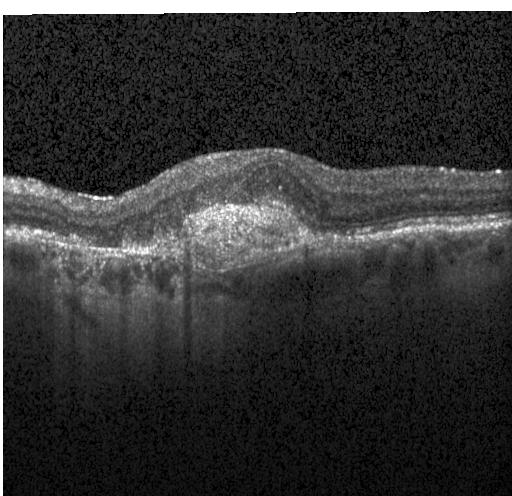

Through the macula. OCT B-scan.
Impression: a choroidal neovascular membrane.